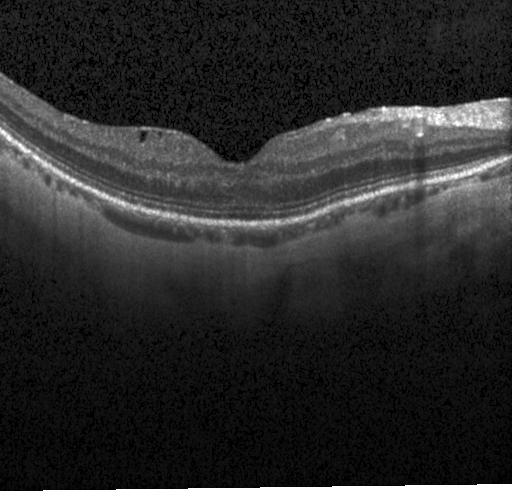
No CNV, DME, or drusen.